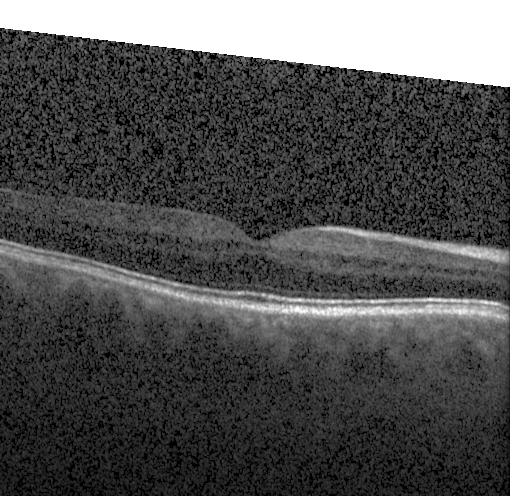
Impression: no evidence of CNV, DME, or drusen.